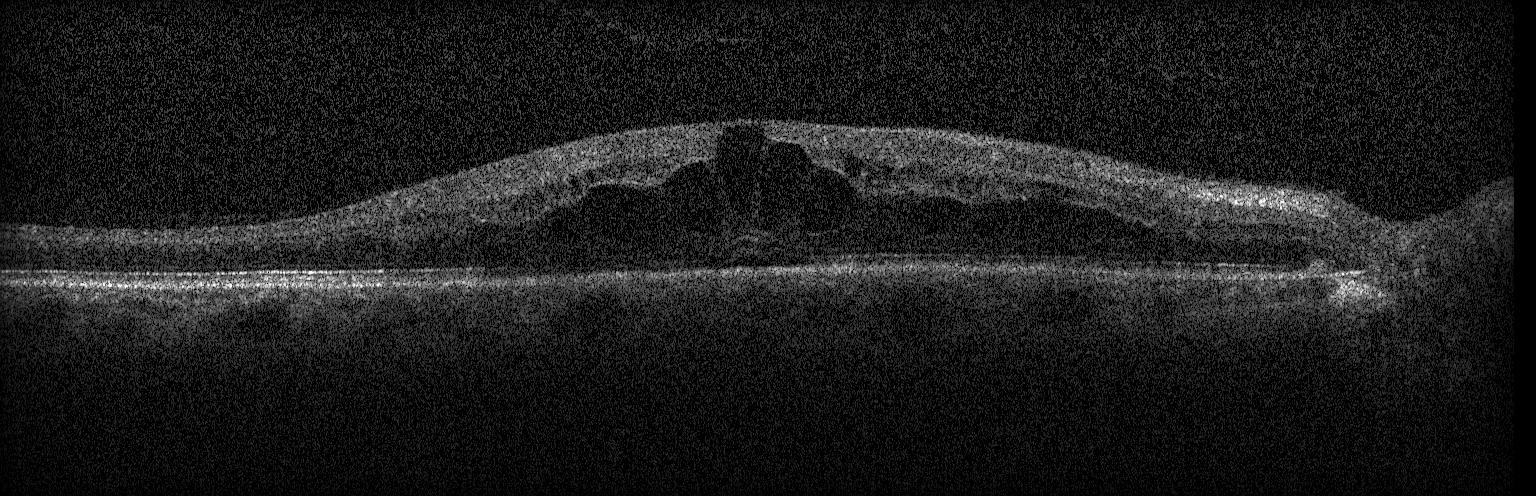
Retinal OCT cross-section, SD-OCT, acquired on a Heidelberg Spectralis. Diagnosis: DME.